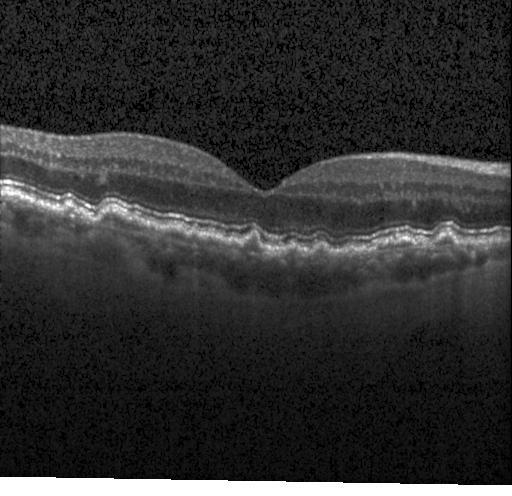
Assessment: multiple drusen.